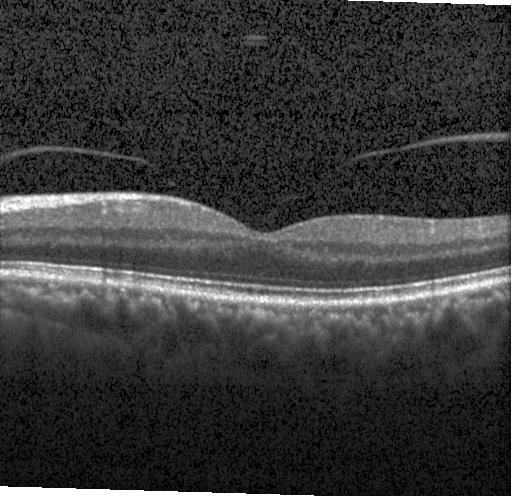
OCT finding: no evidence of CNV, DME, or drusen.